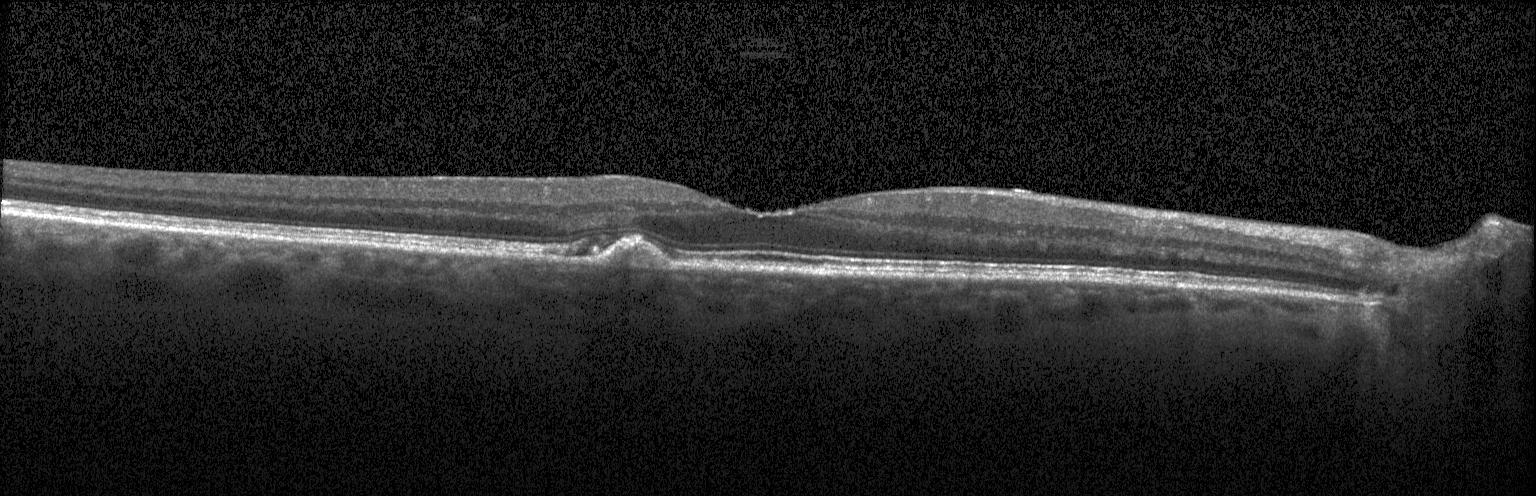

Optical coherence tomography scan, spectral-domain OCT, horizontal scan through the fovea, instrument: Heidelberg Spectralis — Diagnosis: a choroidal neovascular membrane.